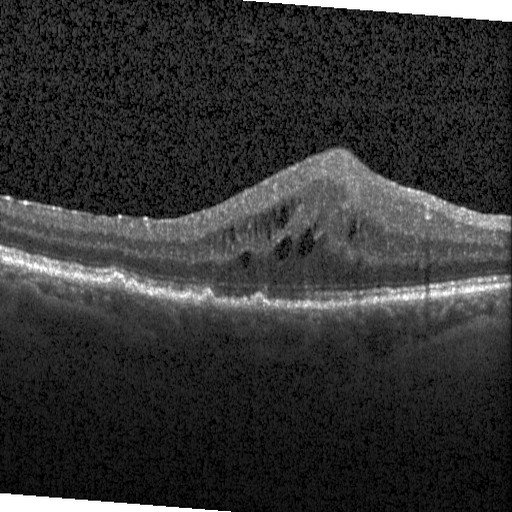

Spectral-domain optical coherence tomography. Acquired on a Heidelberg Spectralis. Macular scan. Optical coherence tomography B-scan. Finding: diabetic macular edema (DME).